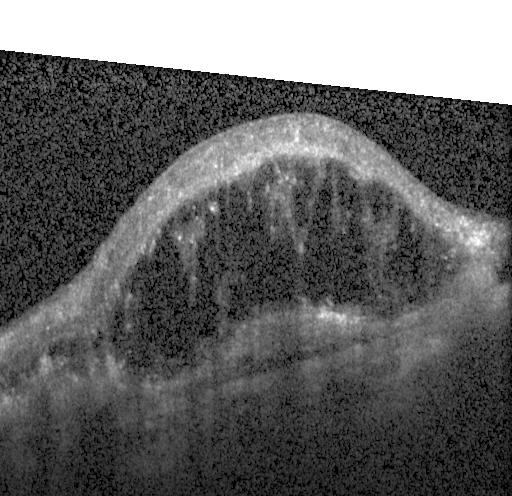
Through the macula · spectral-domain optical coherence tomography · optical coherence tomography scan · acquired on a Heidelberg Spectralis. Assessment: diabetic macular edema.